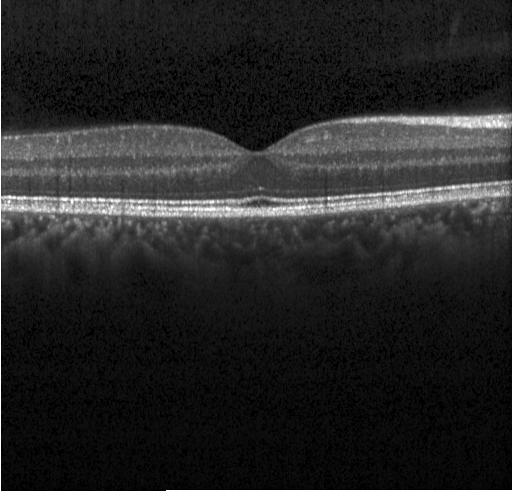

No evidence of choroidal neovascularization, diabetic macular edema, or drusen.